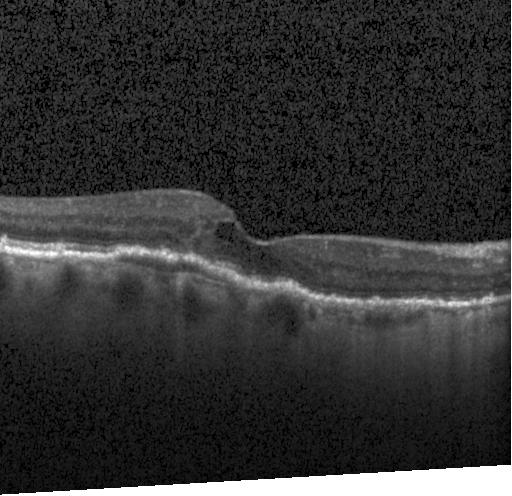
Diagnosis: a choroidal neovascular membrane.